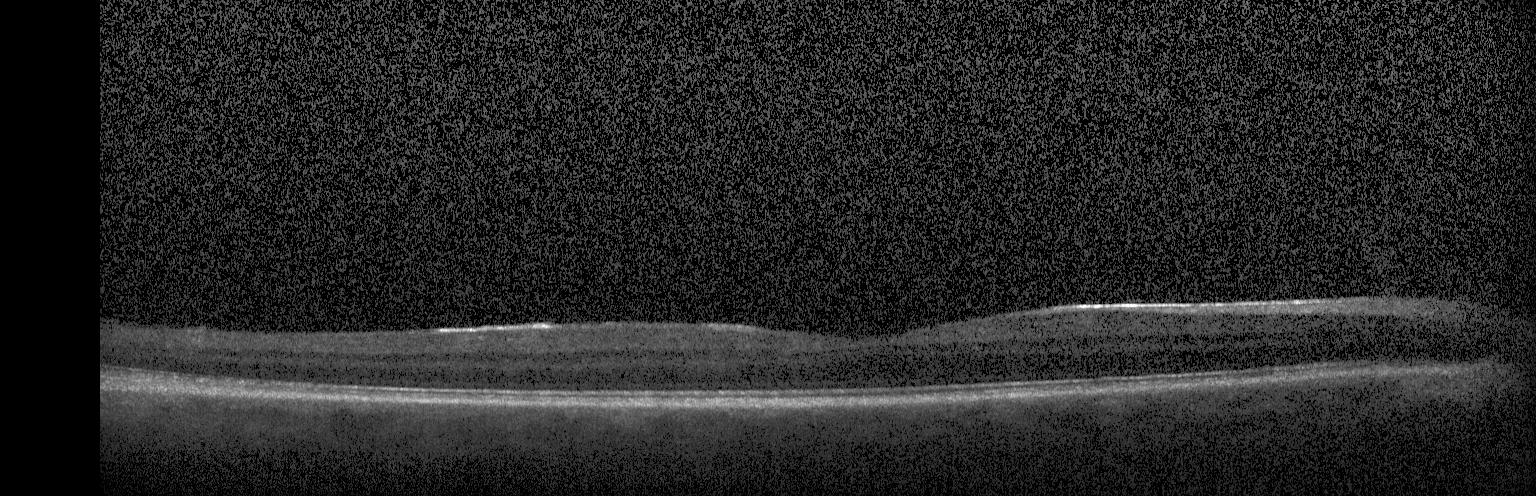
Heidelberg Spectralis OCT system. Through the macula. Optical coherence tomography B-scan. SD-OCT
Impression: no choroidal neovascularization, no diabetic macular edema, and no drusen.